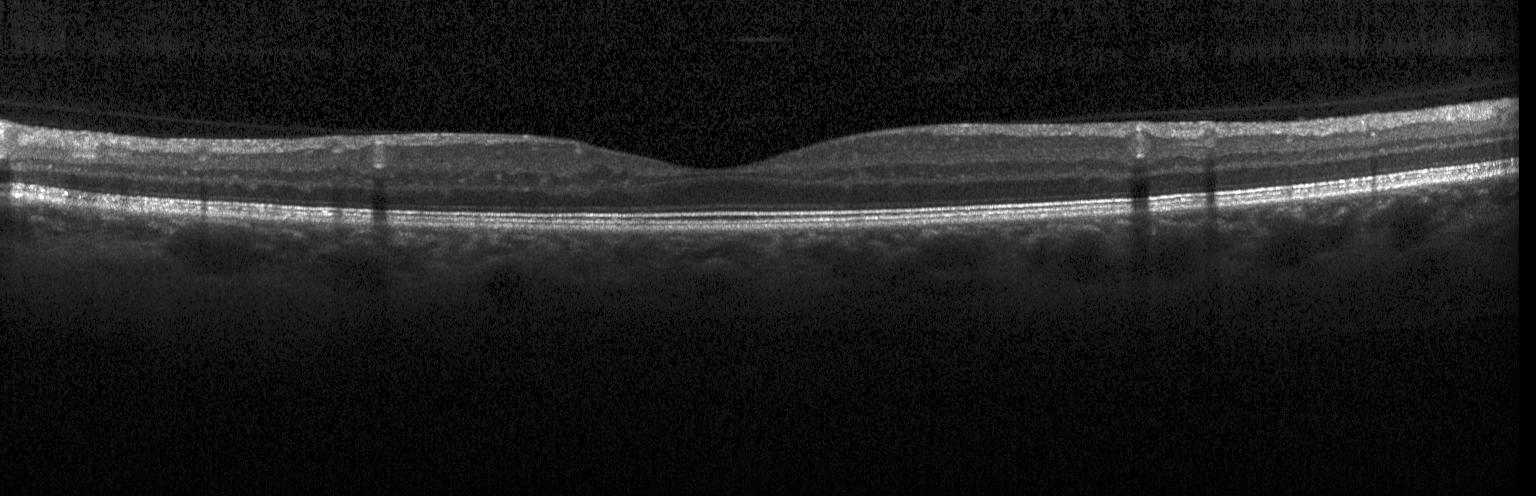
OCT B-scan showing no choroidal neovascularization, diabetic macular edema, or drusen.